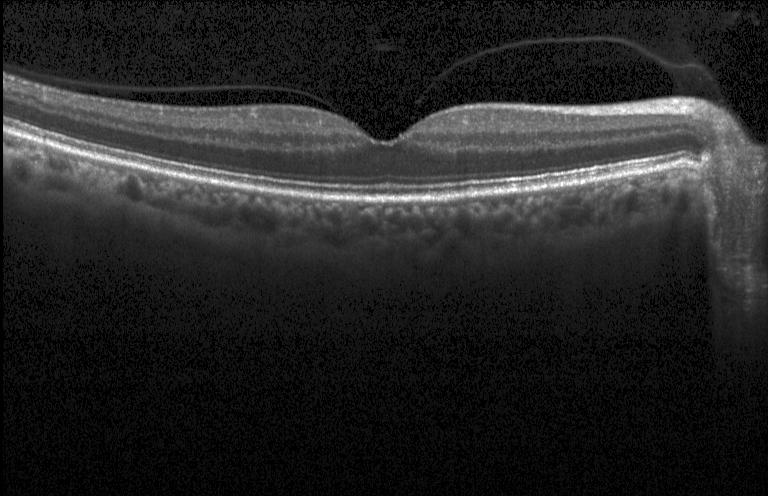

OCT B-scan showing neither CNV, DME, nor drusen.